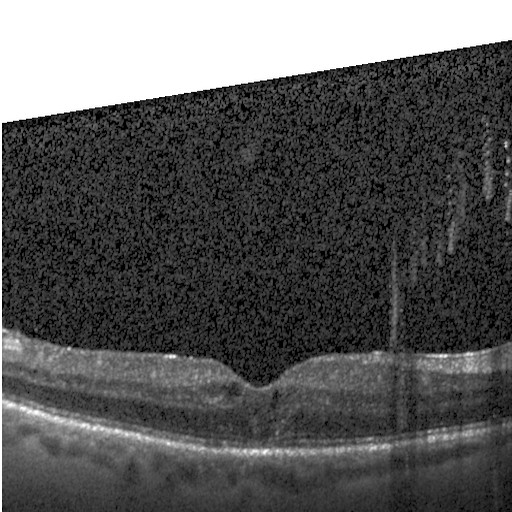

Assessment: diabetic macular edema (DME).